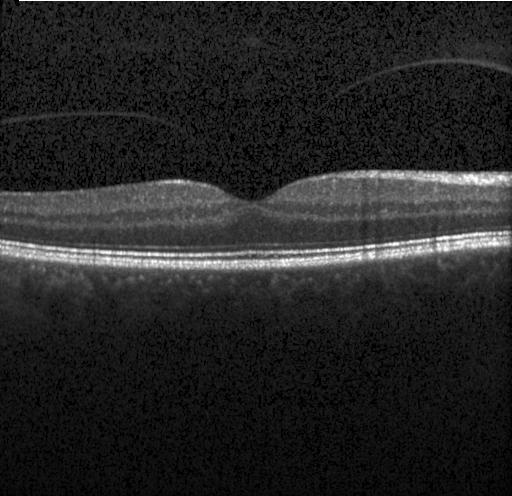
Optical coherence tomography B-scan — The scan shows neither choroidal neovascularization, diabetic macular edema, nor drusen.